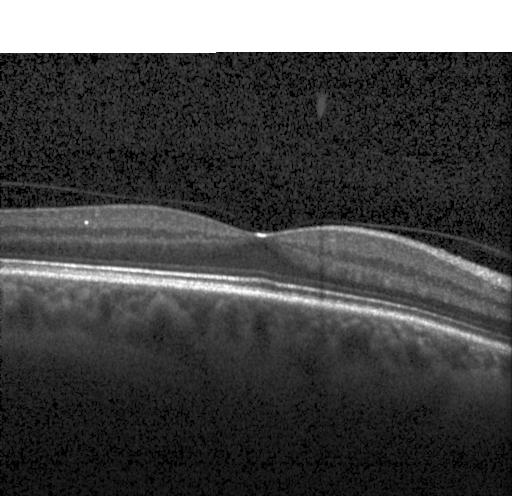
Instrument: Heidelberg Spectralis; macular scan; SD-OCT; OCT line scan
Finding: no choroidal neovascularization, diabetic macular edema, or drusen.